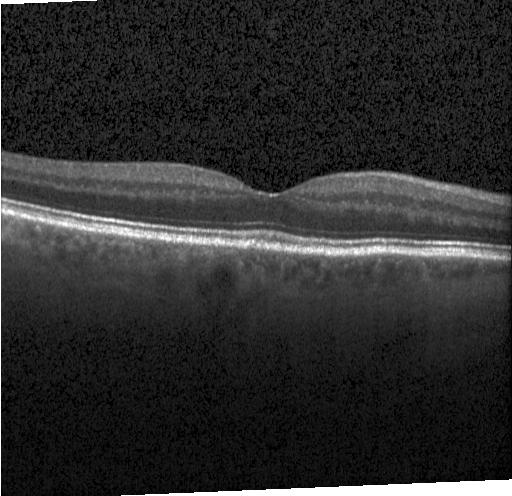

Retinal OCT cross-section.
Diagnosis: no choroidal neovascularization, diabetic macular edema, or drusen.